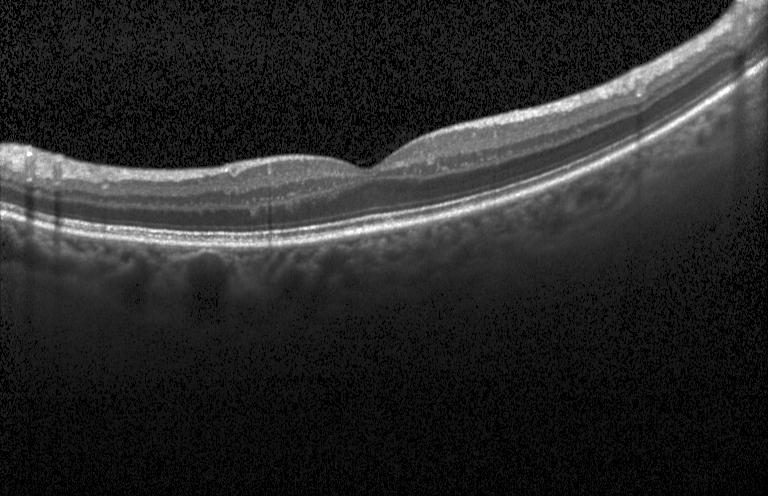 Optical coherence tomography scan.
Impression: no choroidal neovascularization, no diabetic macular edema, and no drusen.